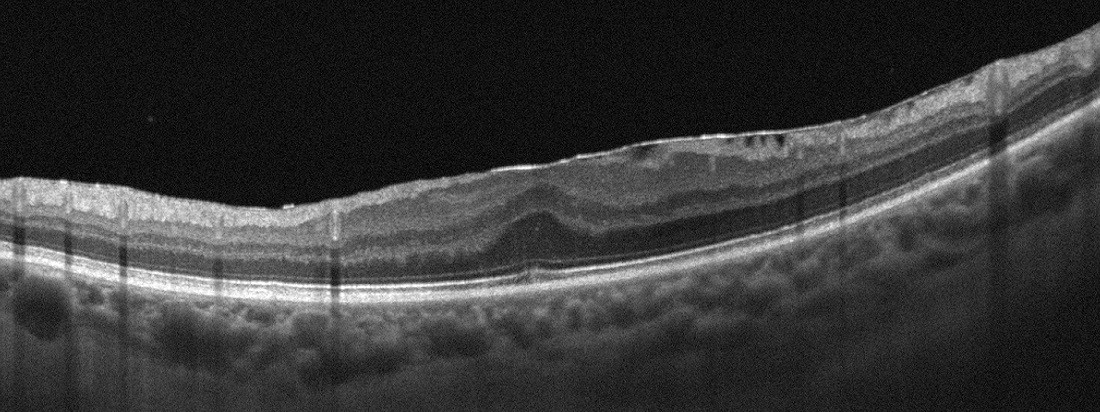
Macular scan. Optovue Avanti RTVue XR. Retinal OCT cross-section
OCT finding: epiretinal membrane (ERM).